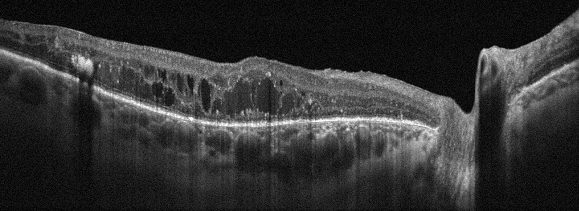
OCT line scan · instrument: Optovue Avanti RTVue XR · OD · through the macula — Diagnosis: diabetic macular edema.